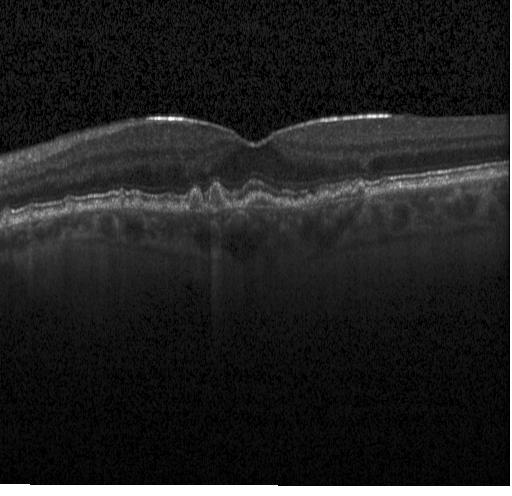
Retinal OCT cross-section showing sub-RPE drusenoid deposits.